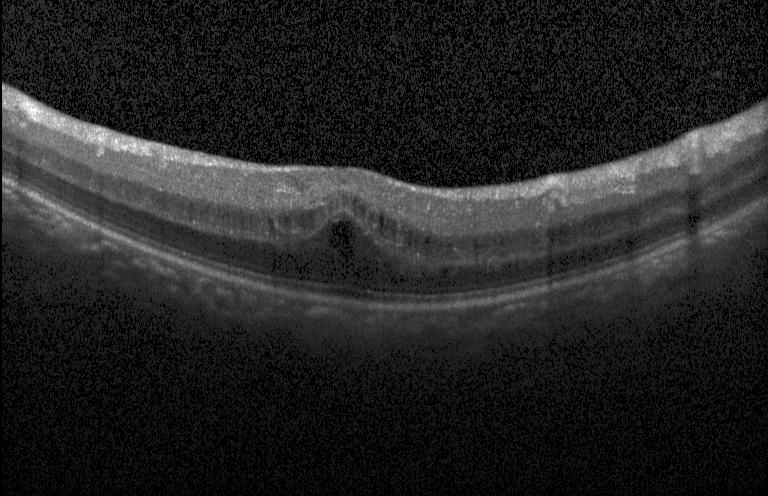
Retinal OCT cross-section.
Macular OCT: diabetic macular edema.